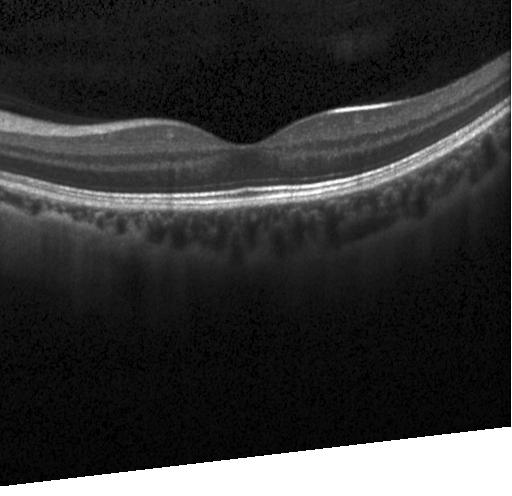 Retinal OCT B-scan · instrument: Heidelberg Spectralis · SD-OCT · through the macula. Macular OCT: no evidence of CNV, DME, or drusen.